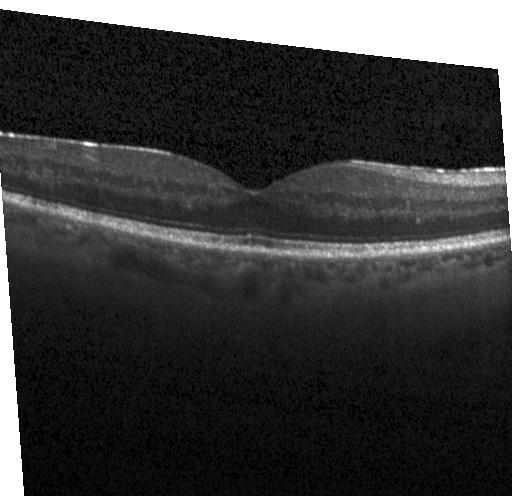 Diagnosis: neither choroidal neovascularization, diabetic macular edema, nor drusen.